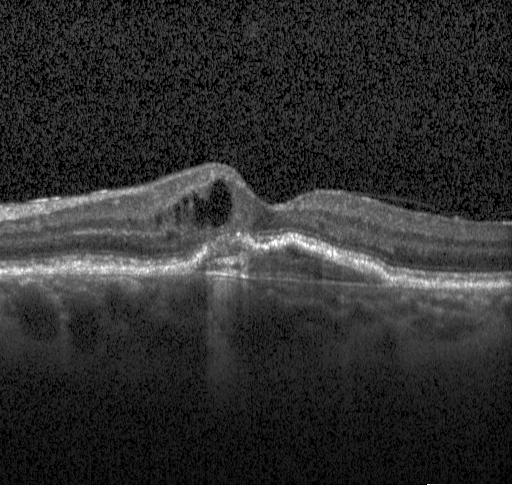
Macular OCT: CNV.